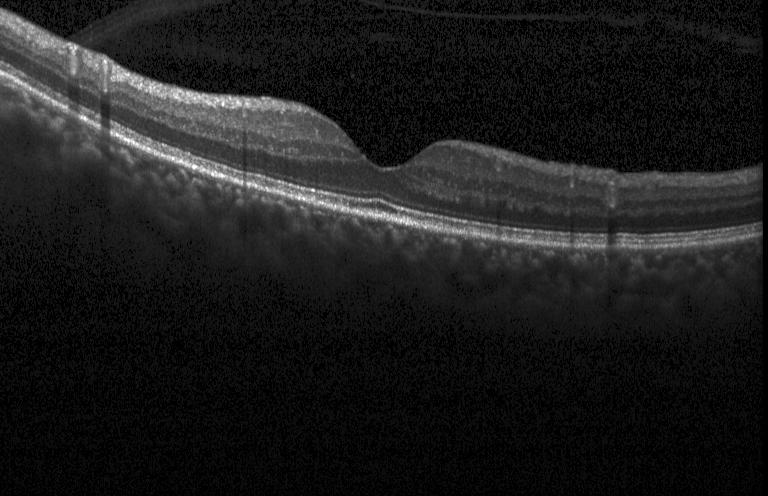 Macular scan, SD-OCT, Heidelberg Spectralis OCT system, OCT B-scan.
OCT finding: neither CNV, DME, nor drusen.